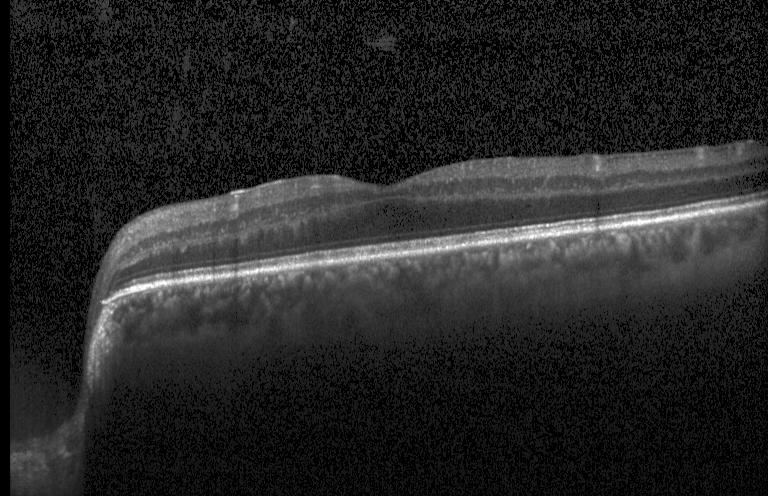
The scan shows no choroidal neovascularization, no diabetic macular edema, and no drusen.